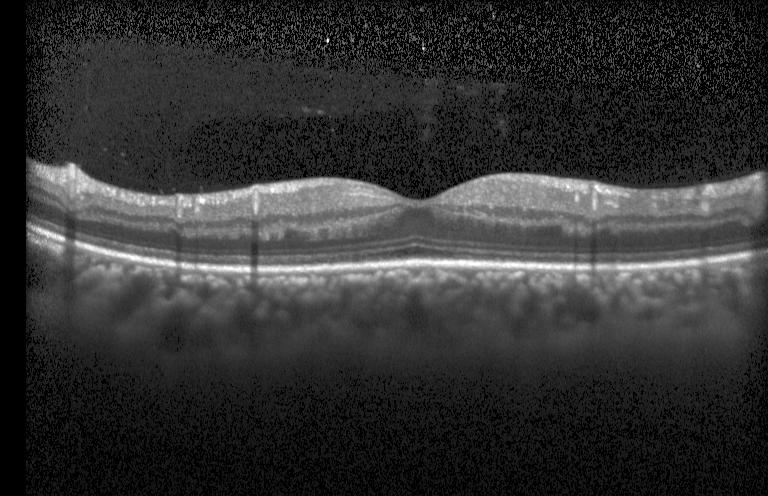

Spectral-domain OCT, OCT line scan
No choroidal neovascularization, diabetic macular edema, or drusen.